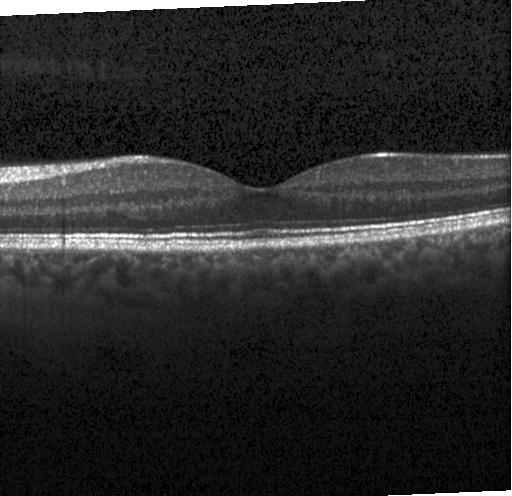

Instrument: Heidelberg Spectralis. Optical coherence tomography B-scan — Finding: no choroidal neovascularization, no diabetic macular edema, and no drusen.